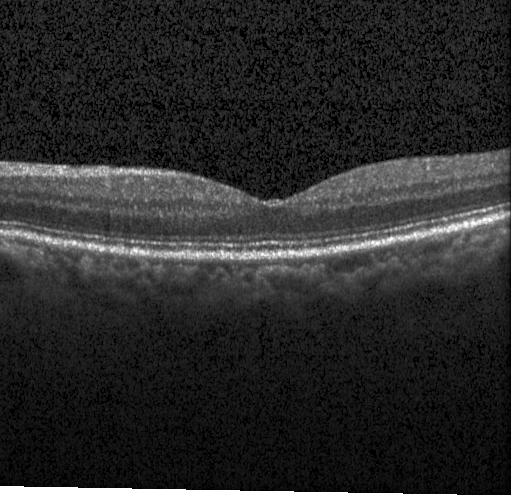 Diagnosis: no choroidal neovascularization, no diabetic macular edema, and no drusen.